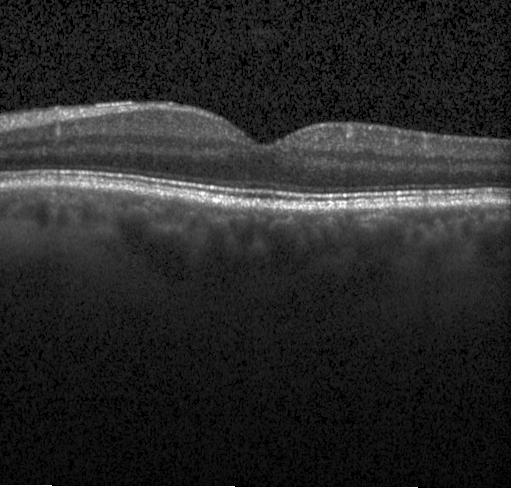

Optical coherence tomography B-scan · centered on the fovea.
This B-scan demonstrates no choroidal neovascularization, diabetic macular edema, or drusen.